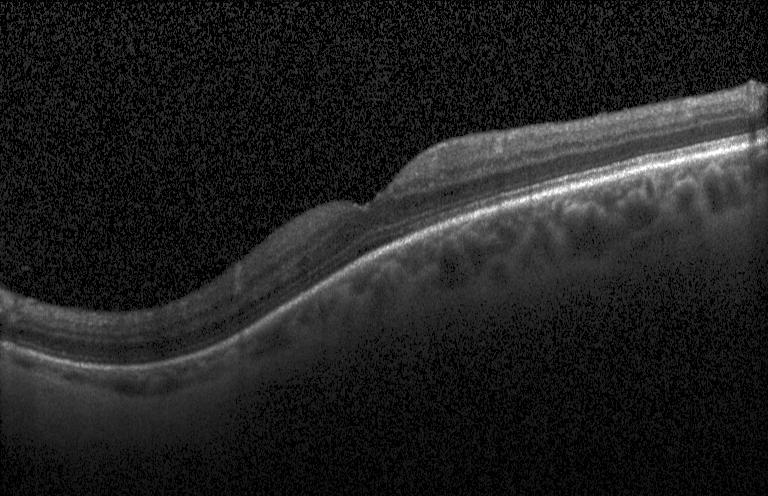

Finding: neither CNV, DME, nor drusen.